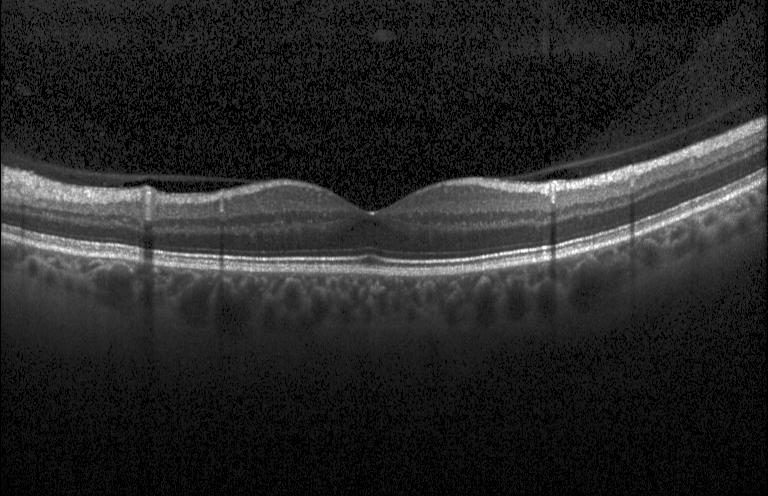
OCT scan showing no evidence of choroidal neovascularization, diabetic macular edema, or drusen.